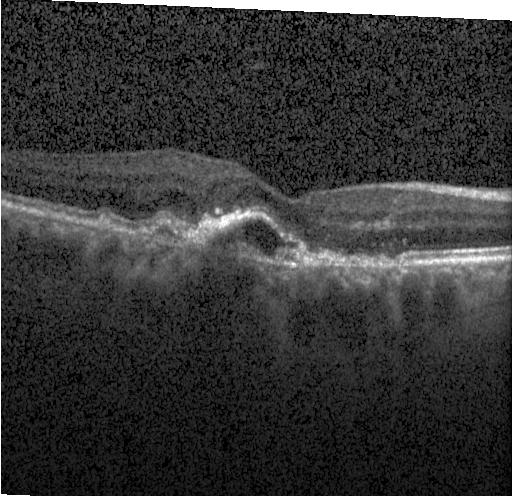

Spectral-domain optical coherence tomography. Fovea-centered. OCT line scan. Heidelberg Spectralis.
Assessment: CNV.